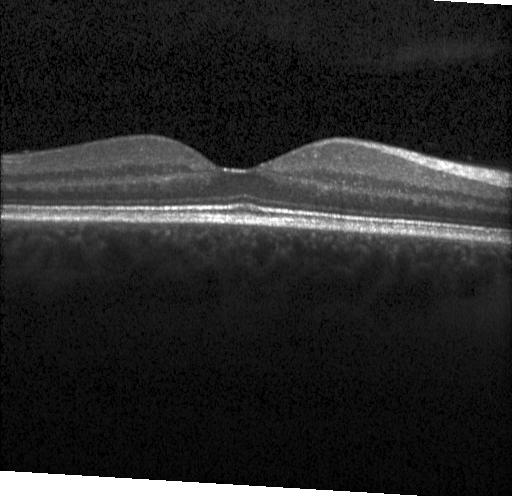 Optical coherence tomography B-scan.
Impression: neither choroidal neovascularization, diabetic macular edema, nor drusen.